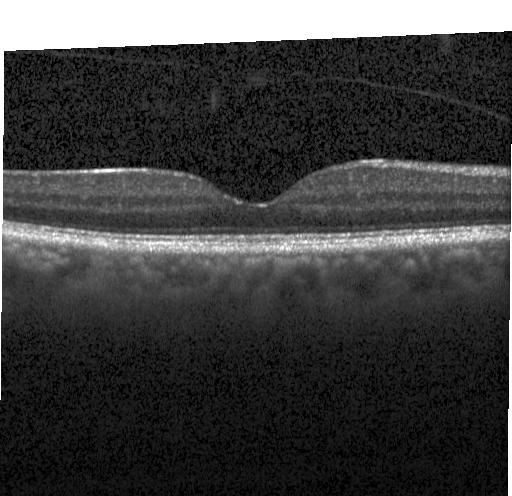

Diagnosis: no choroidal neovascularization, diabetic macular edema, or drusen.